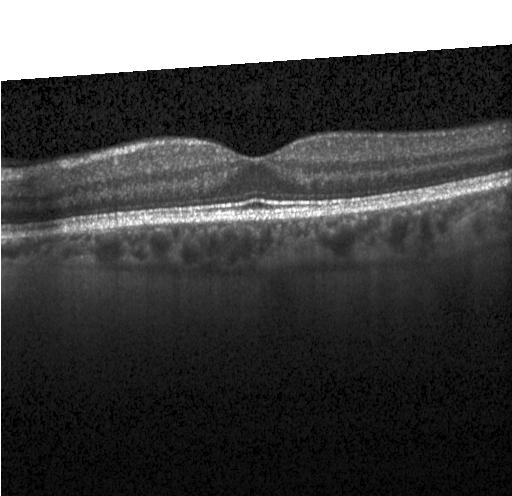

Dx: no choroidal neovascularization, no diabetic macular edema, and no drusen.